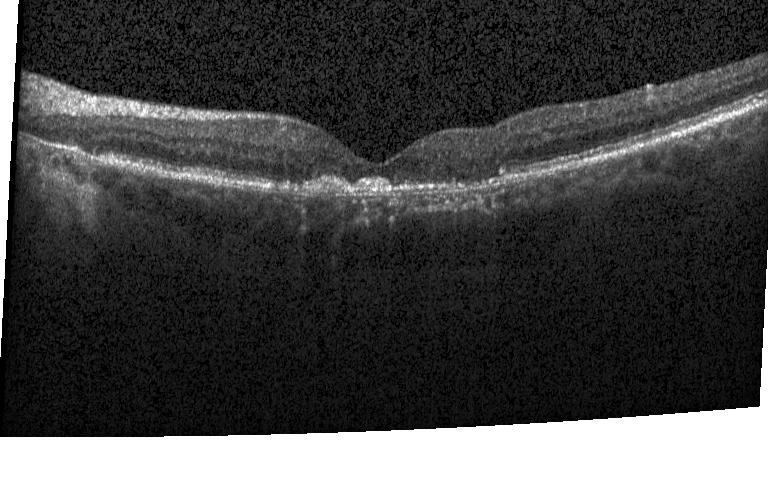

Heidelberg Spectralis OCT system · OCT B-scan
Impression: a choroidal neovascular membrane.